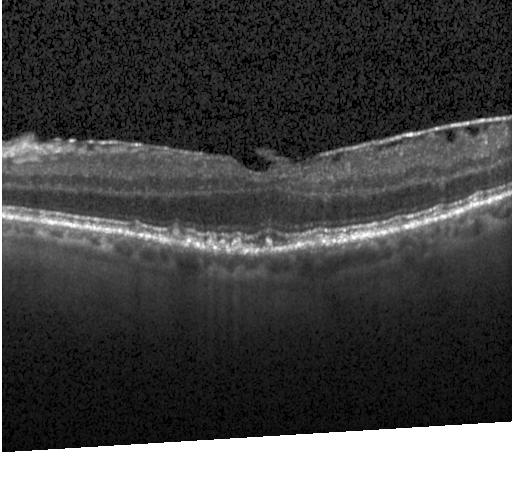
Optical coherence tomography B-scan · centered on the fovea · SD-OCT · Heidelberg Spectralis OCT system — OCT finding: drusen.